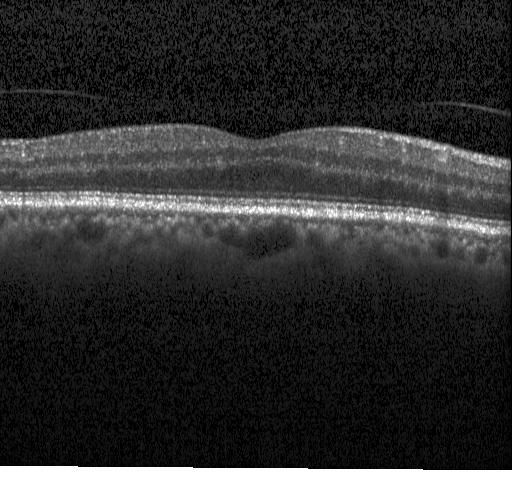
OCT scan showing no evidence of choroidal neovascularization, diabetic macular edema, or drusen.